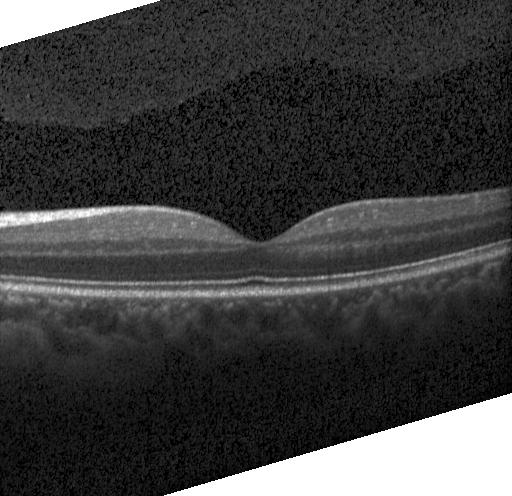 Retinal OCT B-scan
Neither CNV, DME, nor drusen.